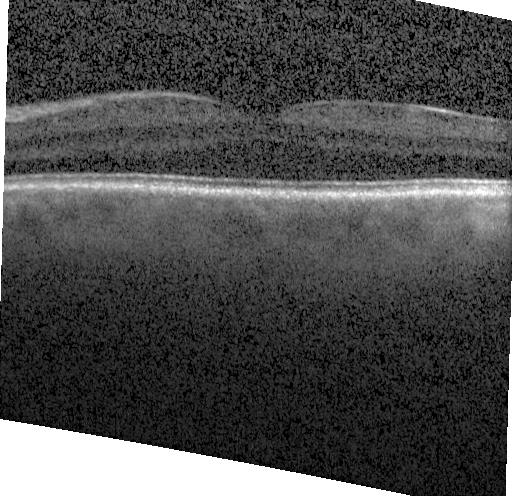

Centered on the fovea. Acquired on a Heidelberg Spectralis. Optical coherence tomography B-scan — Finding: neither choroidal neovascularization, diabetic macular edema, nor drusen.